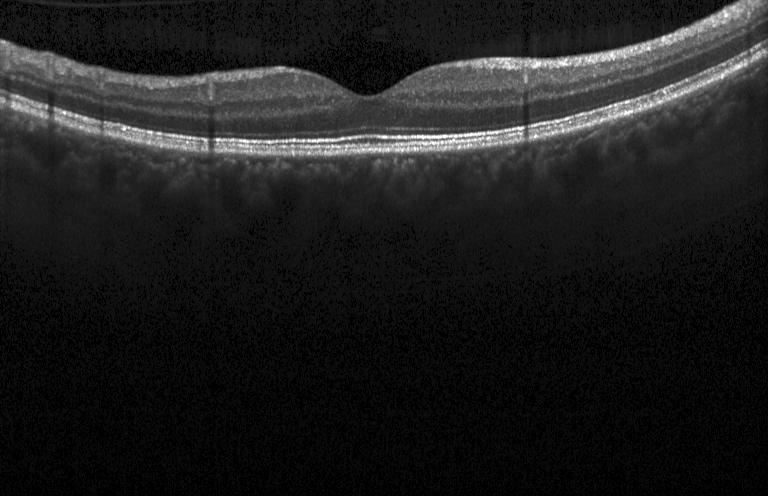

Spectral-domain optical coherence tomography; optical coherence tomography scan; through the macula; Heidelberg Spectralis OCT system.
No choroidal neovascularization, no diabetic macular edema, and no drusen.